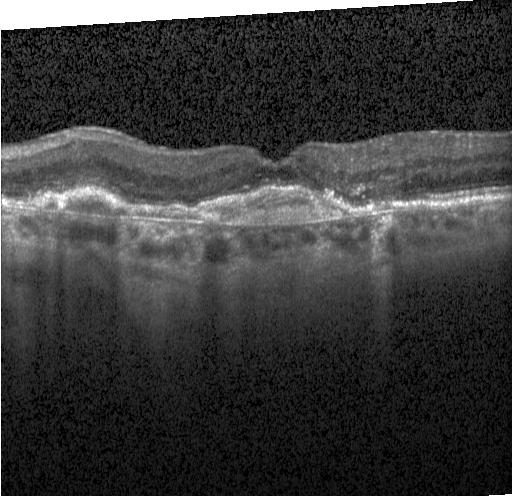
Heidelberg Spectralis OCT system; retinal OCT cross-section — Dx: a choroidal neovascular membrane.